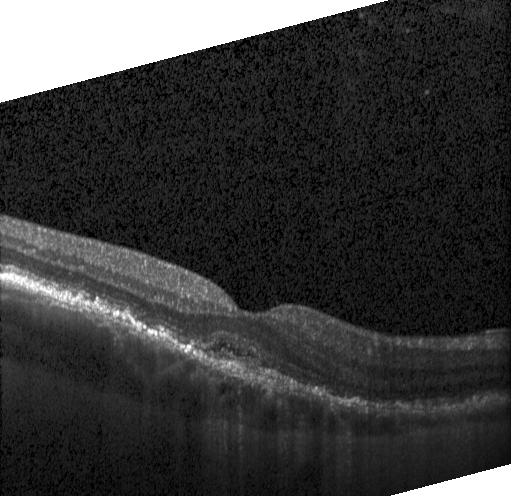
A choroidal neovascular membrane.